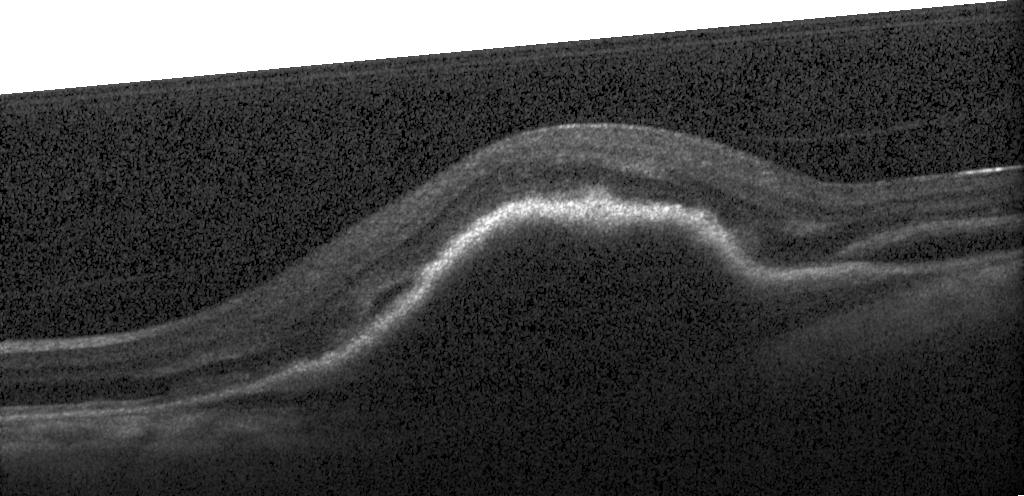

This B-scan demonstrates choroidal neovascularization.